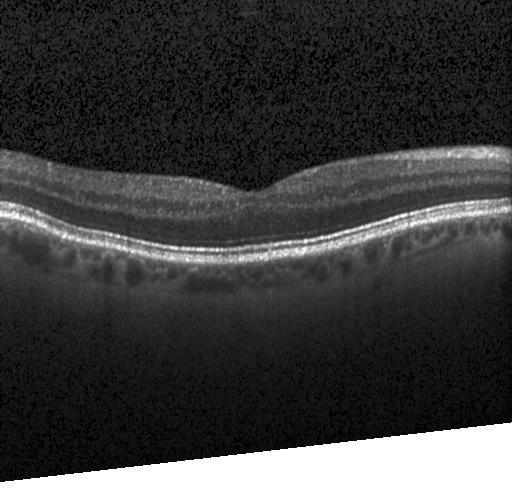

Acquired on a Heidelberg Spectralis; retinal OCT cross-section; spectral-domain OCT; centered on the fovea
Finding: no choroidal neovascularization, diabetic macular edema, or drusen.